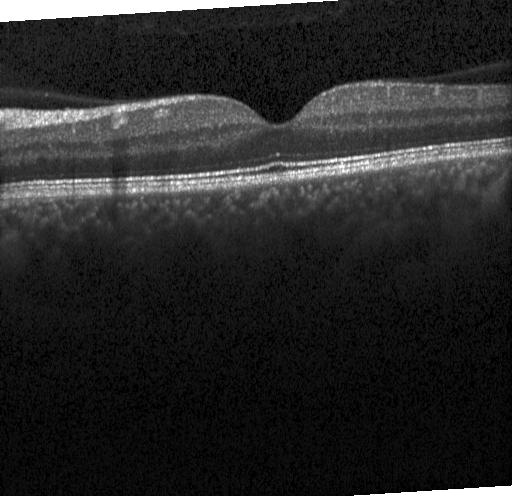

No evidence of choroidal neovascularization, diabetic macular edema, or drusen.